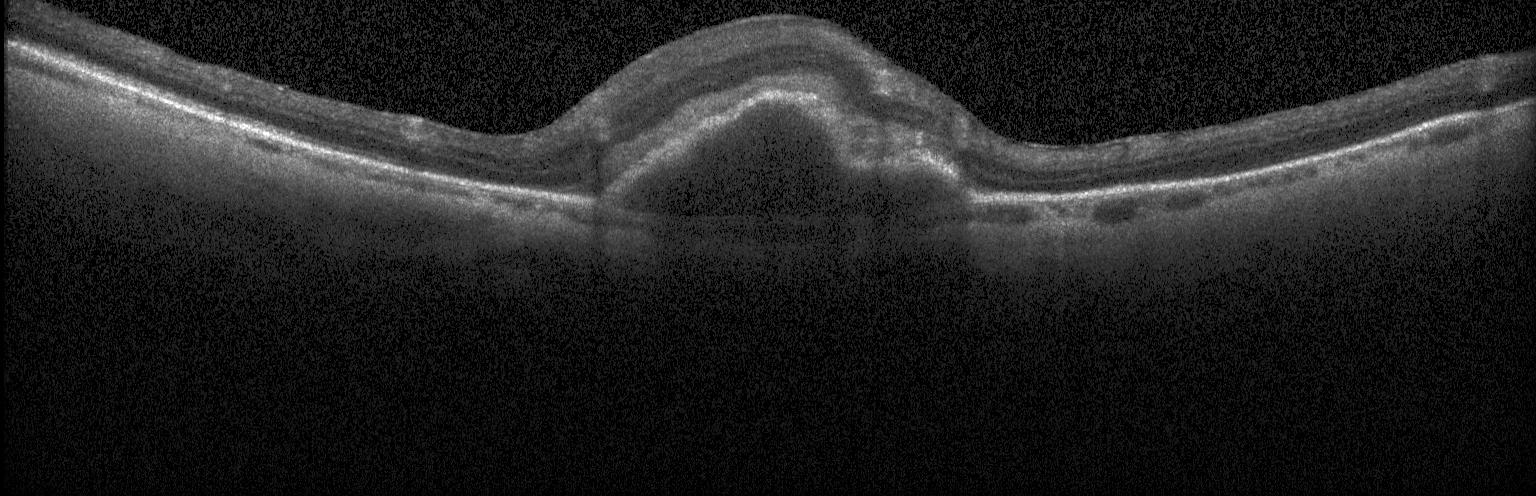

Assessment: CNV.